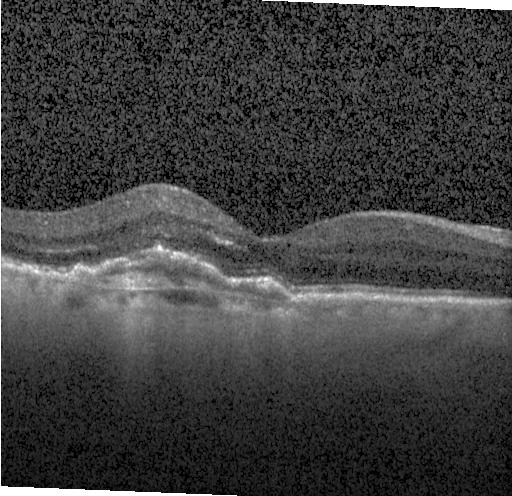

Impression: CNV.